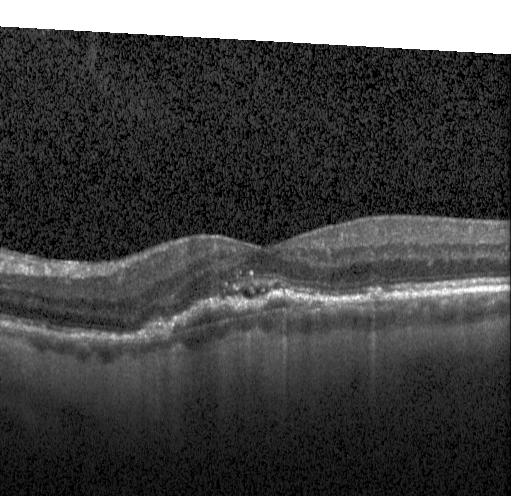

Retinal OCT cross-section showing choroidal neovascularization.